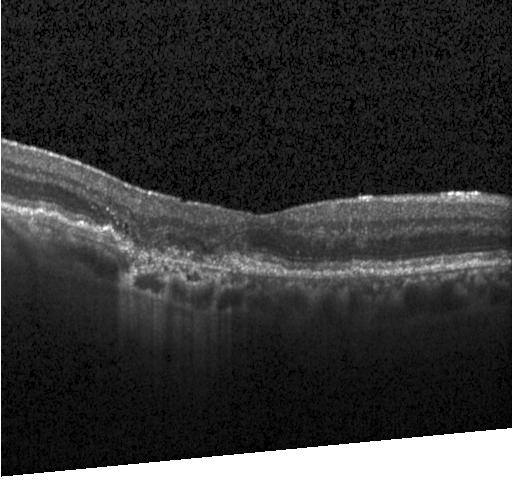 Diagnosis: choroidal neovascularization.